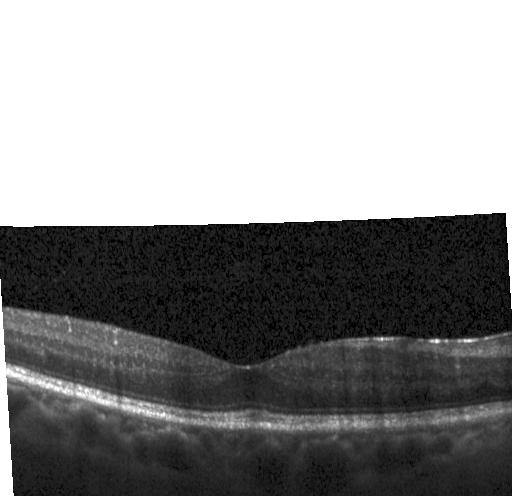 Spectral-domain OCT. Heidelberg Spectralis. OCT B-scan
Diagnosis: no evidence of choroidal neovascularization, diabetic macular edema, or drusen.